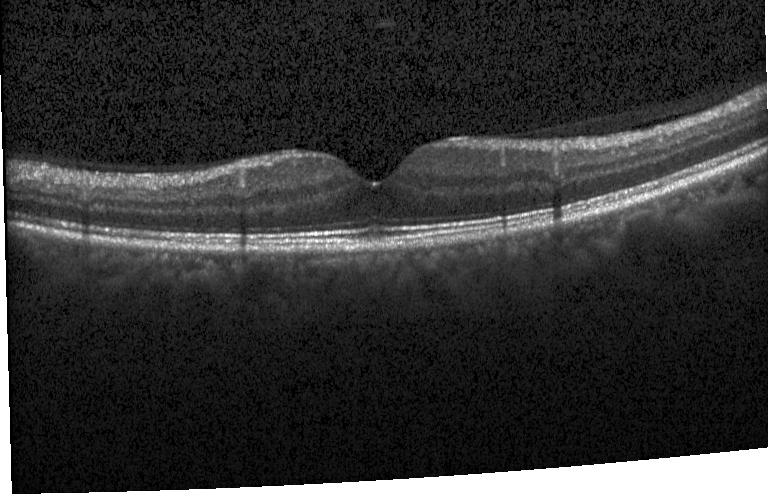 Retinal OCT B-scan
Dx: neither choroidal neovascularization, diabetic macular edema, nor drusen.